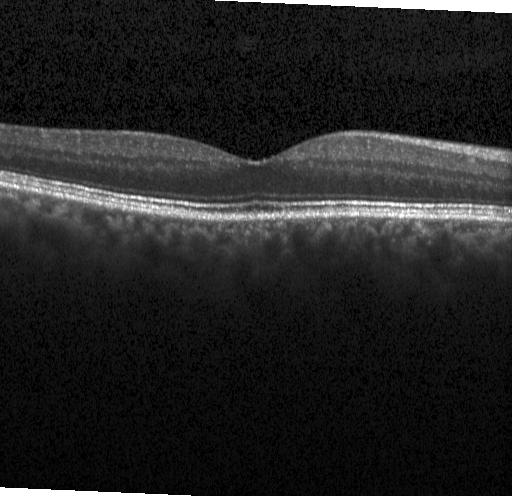
OCT scan showing no choroidal neovascularization, diabetic macular edema, or drusen.